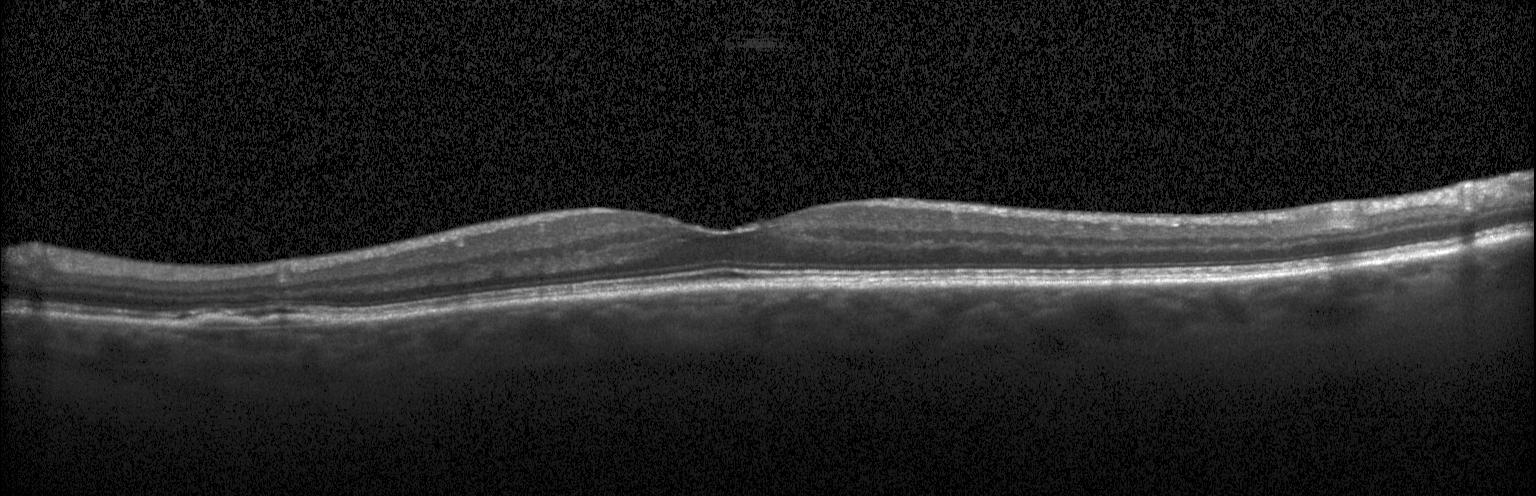
Optical coherence tomography scan · instrument: Heidelberg Spectralis.
The scan shows a choroidal neovascular membrane.